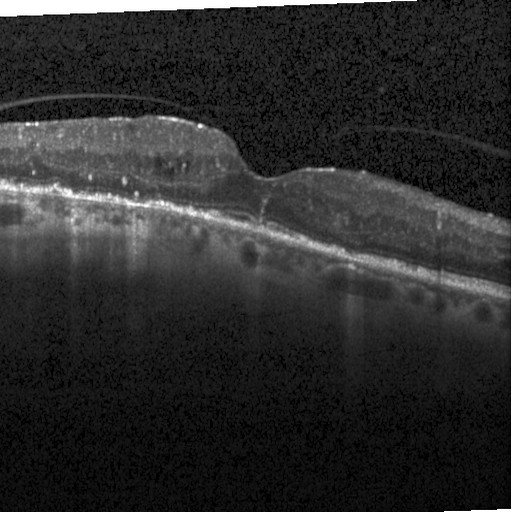

OCT B-scan showing DME.